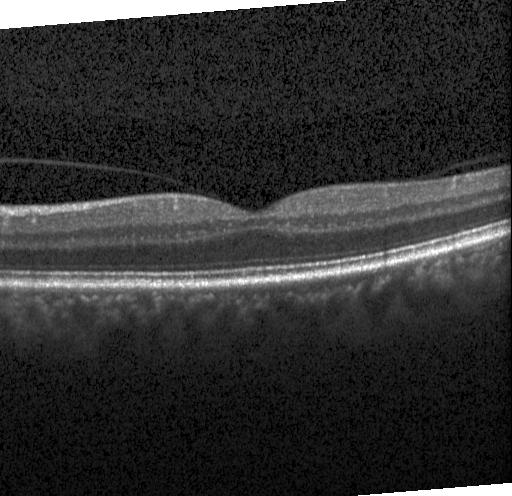 Optical coherence tomography B-scan; instrument: Heidelberg Spectralis — Finding: neither CNV, DME, nor drusen.